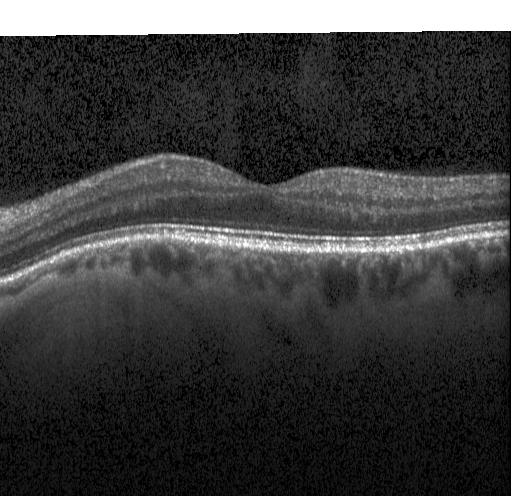

Finding: no evidence of choroidal neovascularization, diabetic macular edema, or drusen.